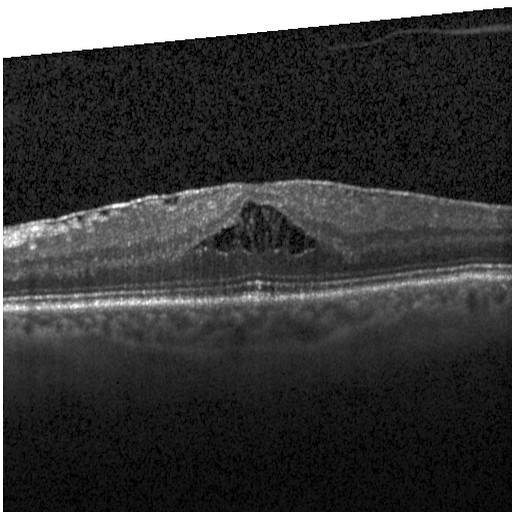 Horizontal scan through the fovea · Heidelberg Spectralis OCT system · OCT line scan · SD-OCT. Diagnosis: DME.